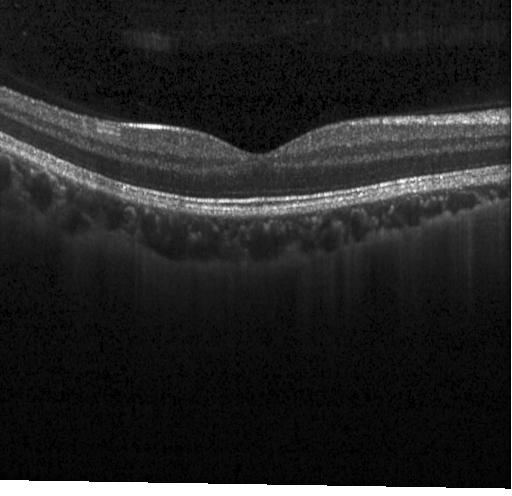
Horizontal scan through the fovea · OCT line scan. Impression: no evidence of choroidal neovascularization, diabetic macular edema, or drusen.